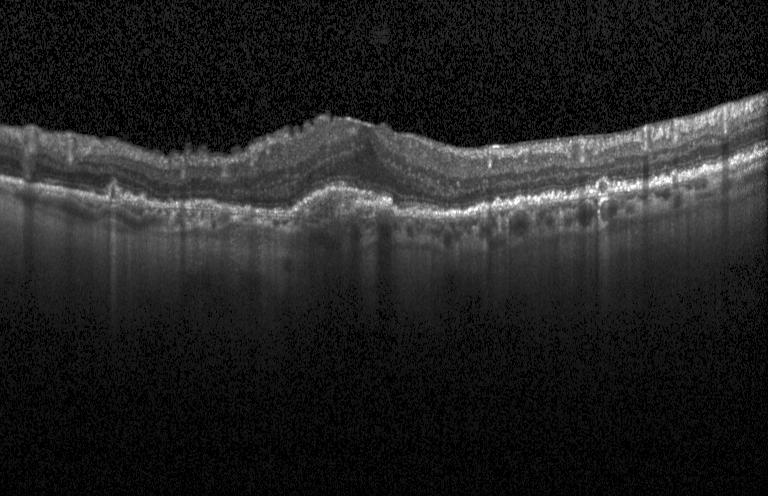

Through the macula · retinal OCT B-scan. This B-scan demonstrates a choroidal neovascular membrane.